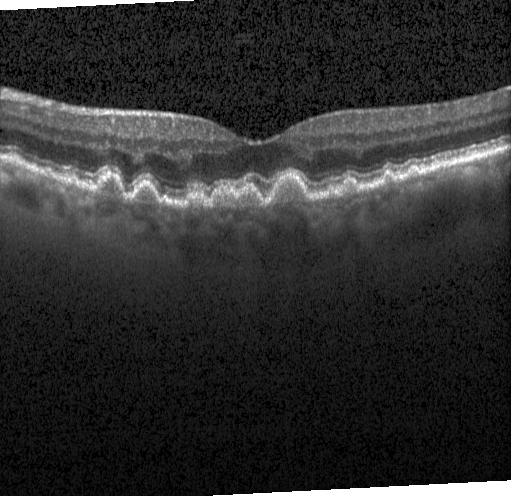
SD-OCT · acquired on a Heidelberg Spectralis · optical coherence tomography scan · fovea-centered. Assessment: sub-RPE drusenoid deposits.